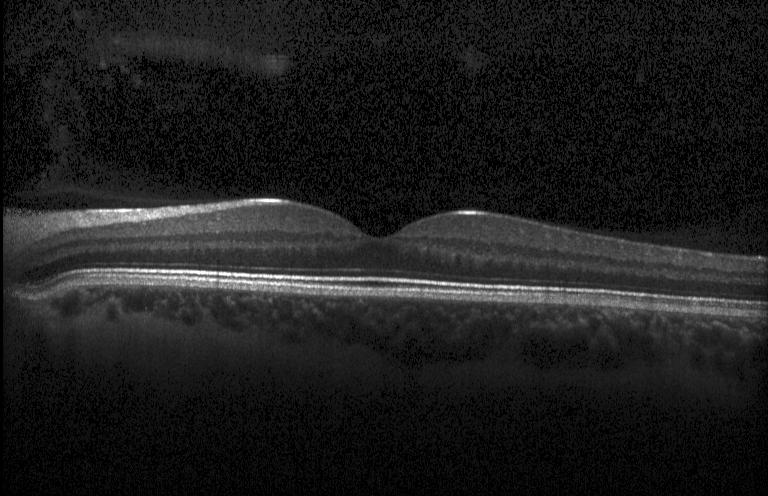 OCT B-scan; spectral-domain optical coherence tomography; Heidelberg Spectralis; centered on the fovea.
Diagnosis: no CNV, no DME, and no drusen.